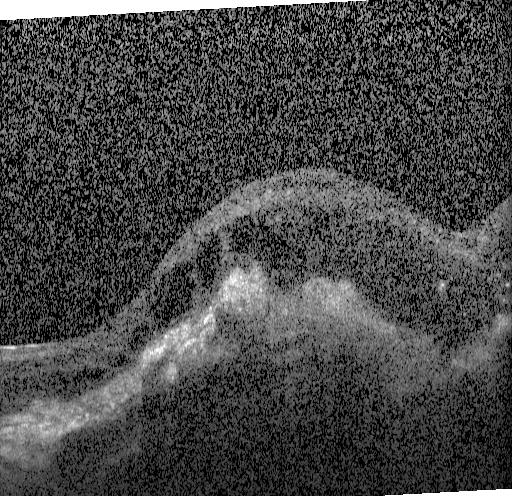
OCT B-scan.
Choroidal neovascularization (CNV).